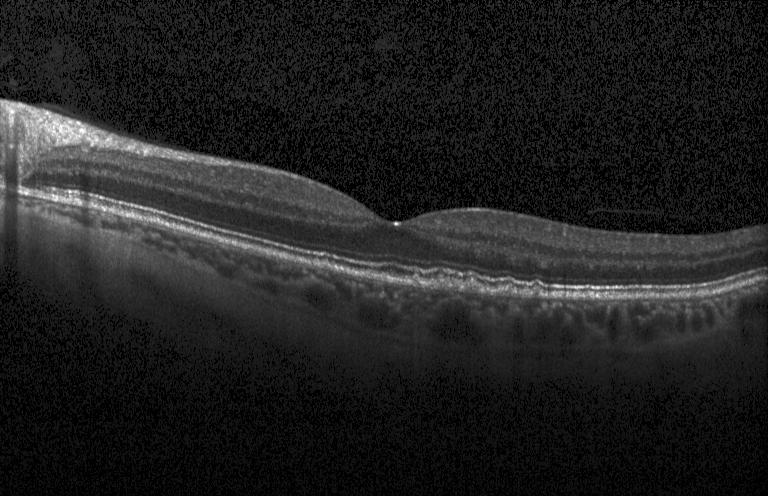
Impression: sub-RPE drusenoid deposits.